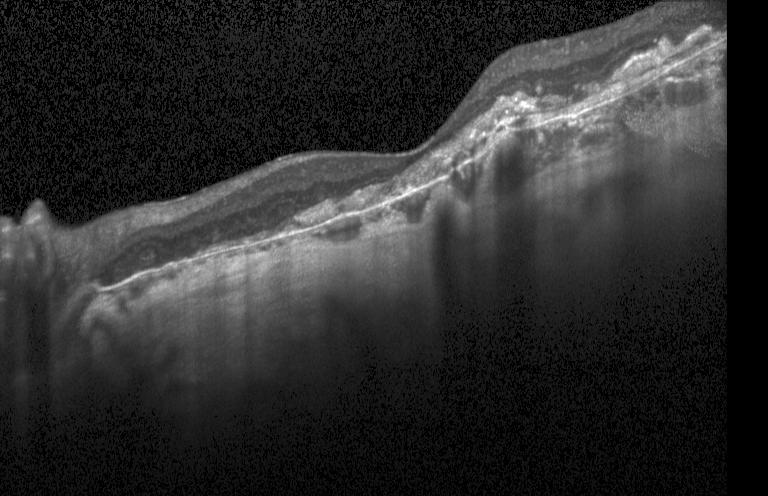
Finding: choroidal neovascularization.